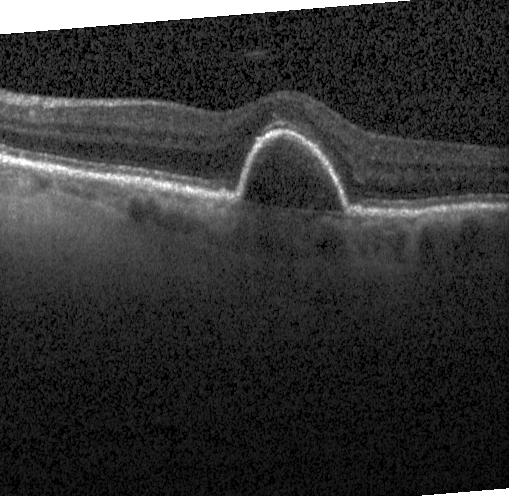

Optical coherence tomography scan; through the macula; spectral-domain OCT; instrument: Heidelberg Spectralis
Dx: a choroidal neovascular membrane.